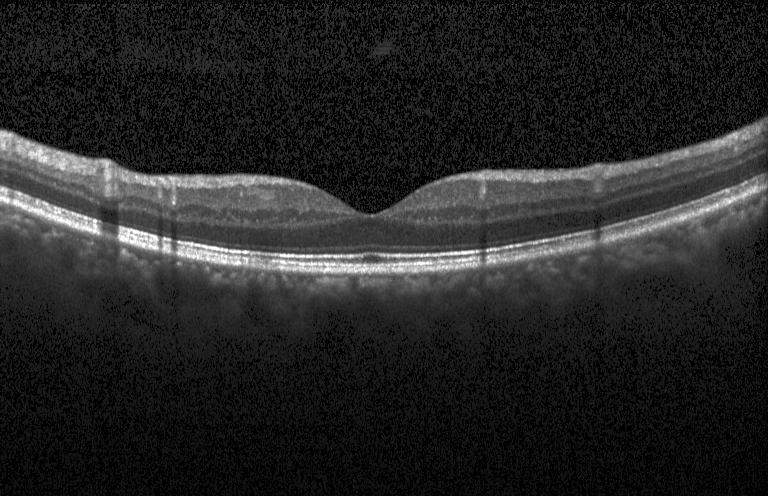 Finding: no CNV, DME, or drusen.